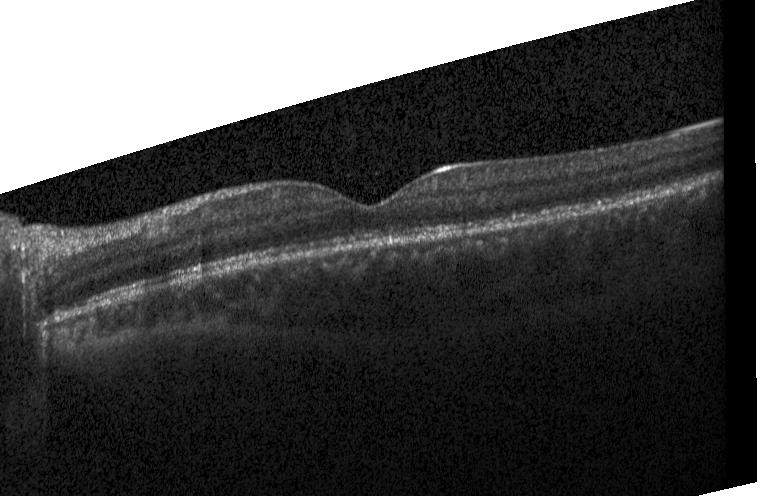
Retinal OCT cross-section; horizontal scan through the fovea; SD-OCT — Dx: neither choroidal neovascularization, diabetic macular edema, nor drusen.